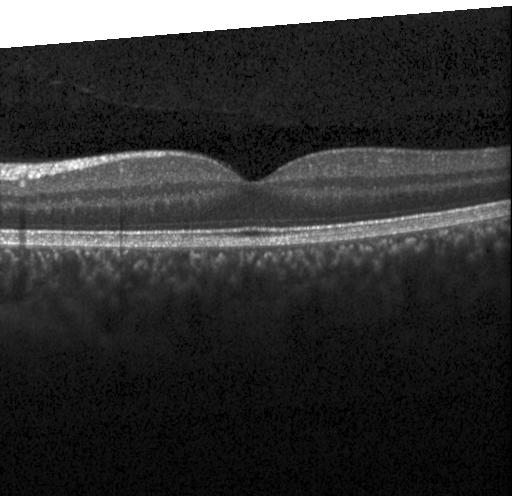 Spectral-domain OCT; Heidelberg Spectralis; optical coherence tomography scan
Impression: neither CNV, DME, nor drusen.